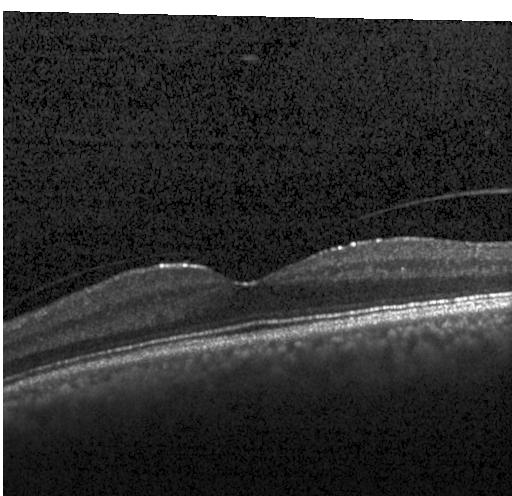
Impression: no evidence of choroidal neovascularization, diabetic macular edema, or drusen.